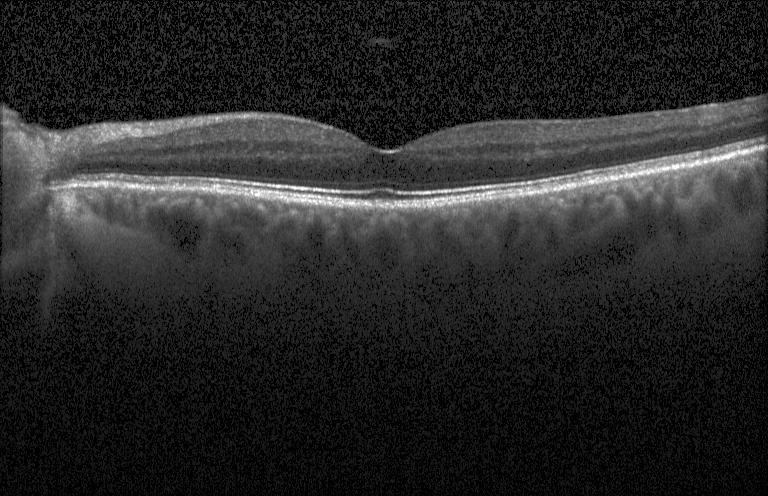
Optical coherence tomography scan · fovea-centered · spectral-domain OCT — Assessment: no choroidal neovascularization, diabetic macular edema, or drusen.